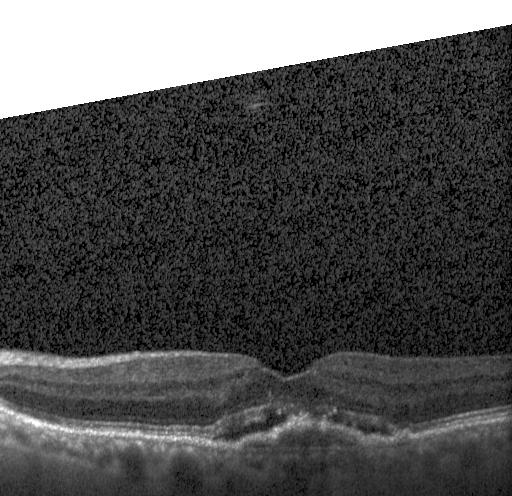
OCT finding: a choroidal neovascular membrane.